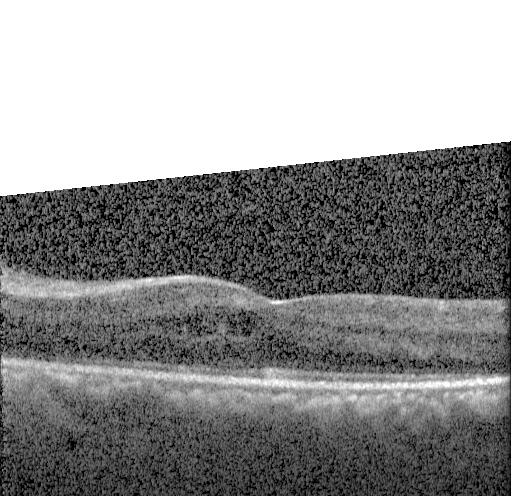
SD-OCT, Heidelberg Spectralis OCT system, retinal OCT B-scan — The scan shows diabetic macular edema.